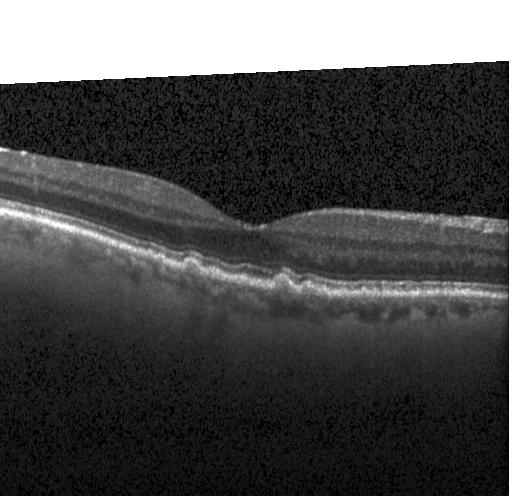 Fovea-centered · acquired on a Heidelberg Spectralis · spectral-domain optical coherence tomography · OCT B-scan.
Finding: sub-RPE drusenoid deposits.